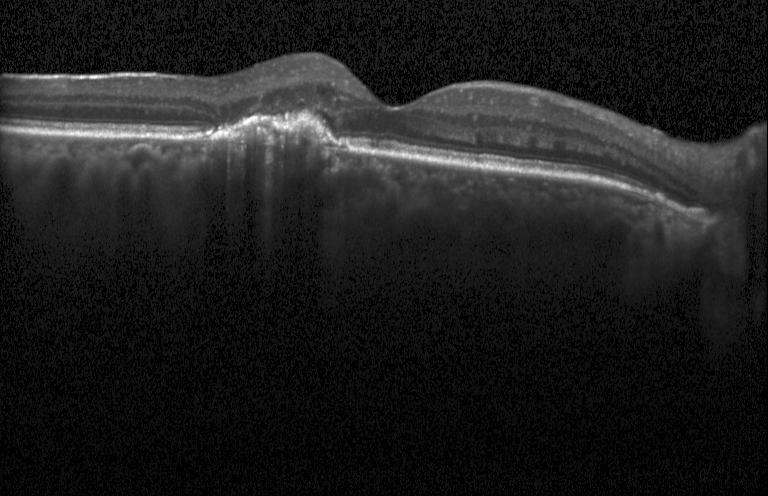
Diagnosis: a choroidal neovascular membrane.